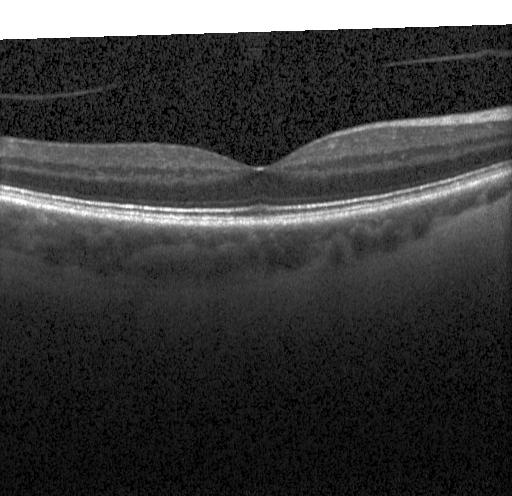

Heidelberg Spectralis OCT system, retinal OCT B-scan, macular scan, SD-OCT. Diagnosis: no choroidal neovascularization, diabetic macular edema, or drusen.